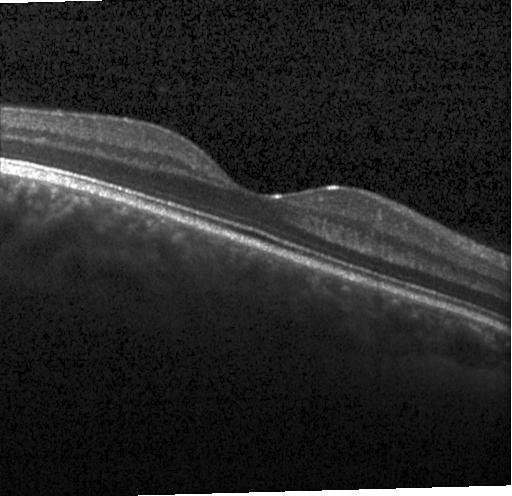

Optical coherence tomography scan, centered on the fovea. The scan shows no choroidal neovascularization, diabetic macular edema, or drusen.